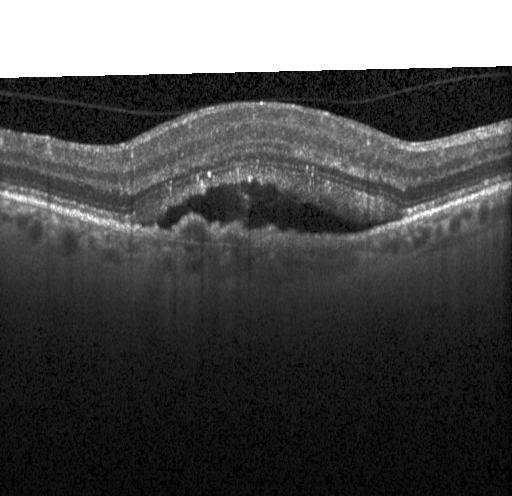

OCT B-scan
This B-scan demonstrates a choroidal neovascular membrane.